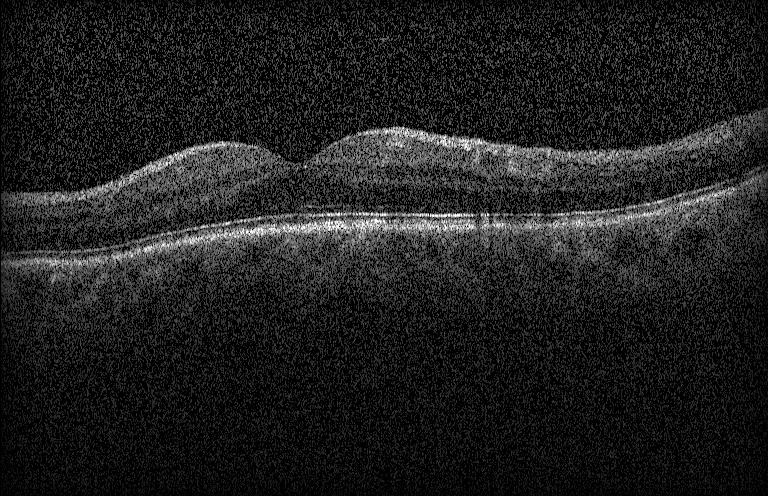
SD-OCT; fovea-centered; retinal OCT cross-section — Diagnosis: no evidence of CNV, DME, or drusen.